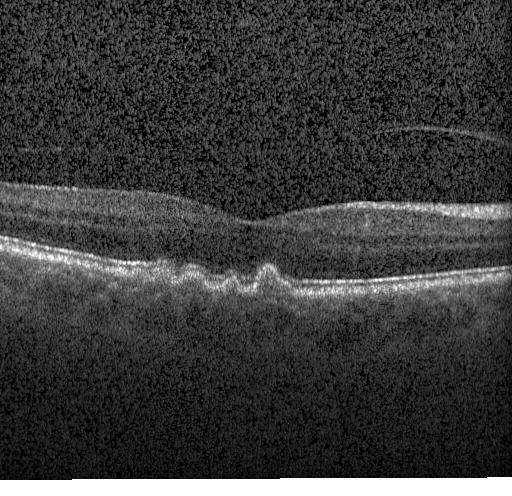
Heidelberg Spectralis OCT system. OCT B-scan. Through the macula. Spectral-domain OCT. OCT finding: drusen.